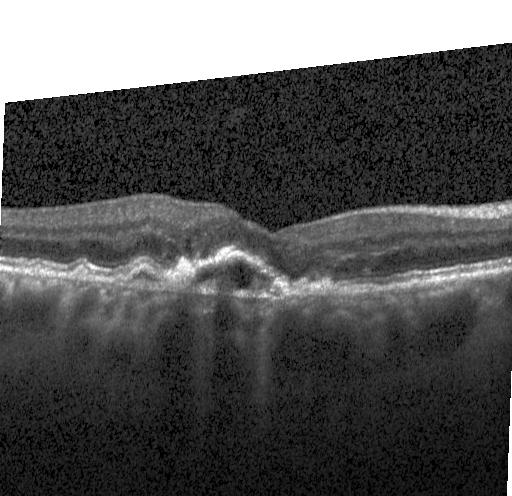 Macular OCT demonstrating choroidal neovascularization (CNV).